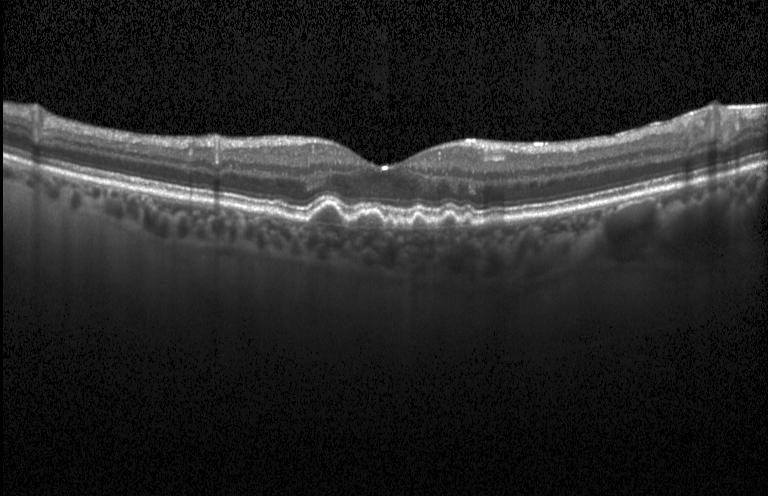

OCT line scan
Sub-RPE drusenoid deposits.